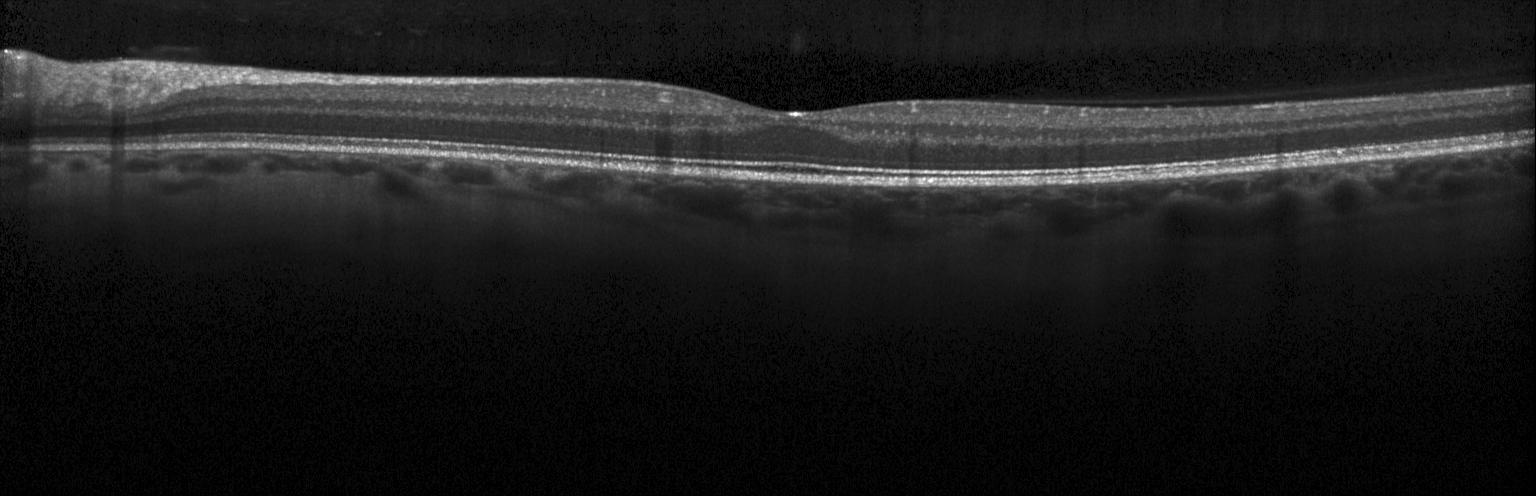

SD-OCT, instrument: Heidelberg Spectralis, OCT line scan, through the macula — OCT finding: no evidence of choroidal neovascularization, diabetic macular edema, or drusen.